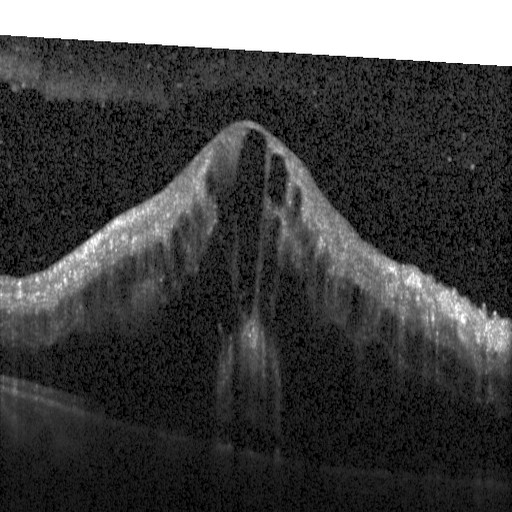
Finding: diabetic macular edema (DME).